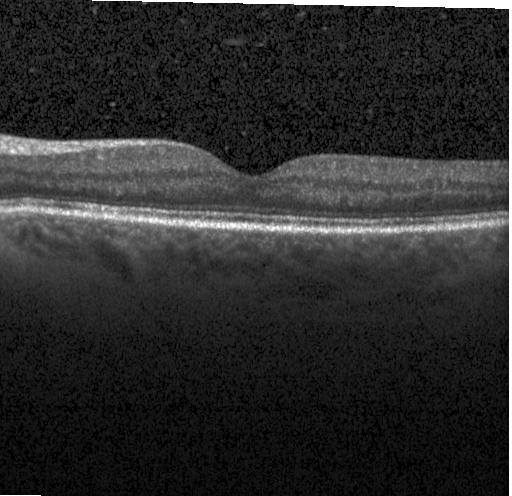
Macular OCT demonstrating no CNV, no DME, and no drusen.